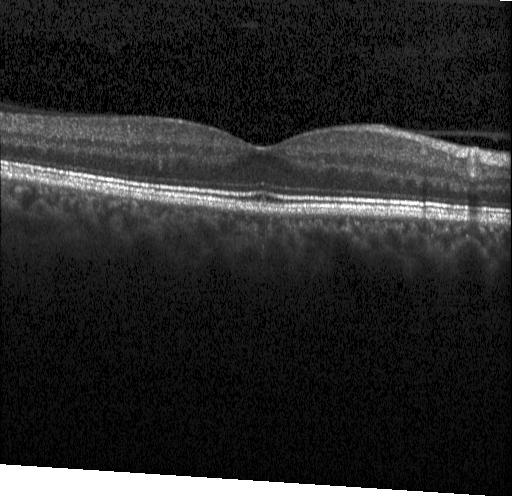
Retinal OCT cross-section
The scan shows neither CNV, DME, nor drusen.